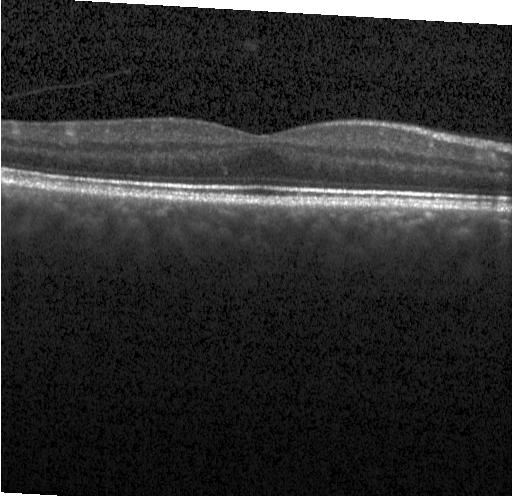
Spectral-domain OCT, horizontal scan through the fovea, acquired on a Heidelberg Spectralis, retinal OCT cross-section — Finding: no CNV, no DME, and no drusen.